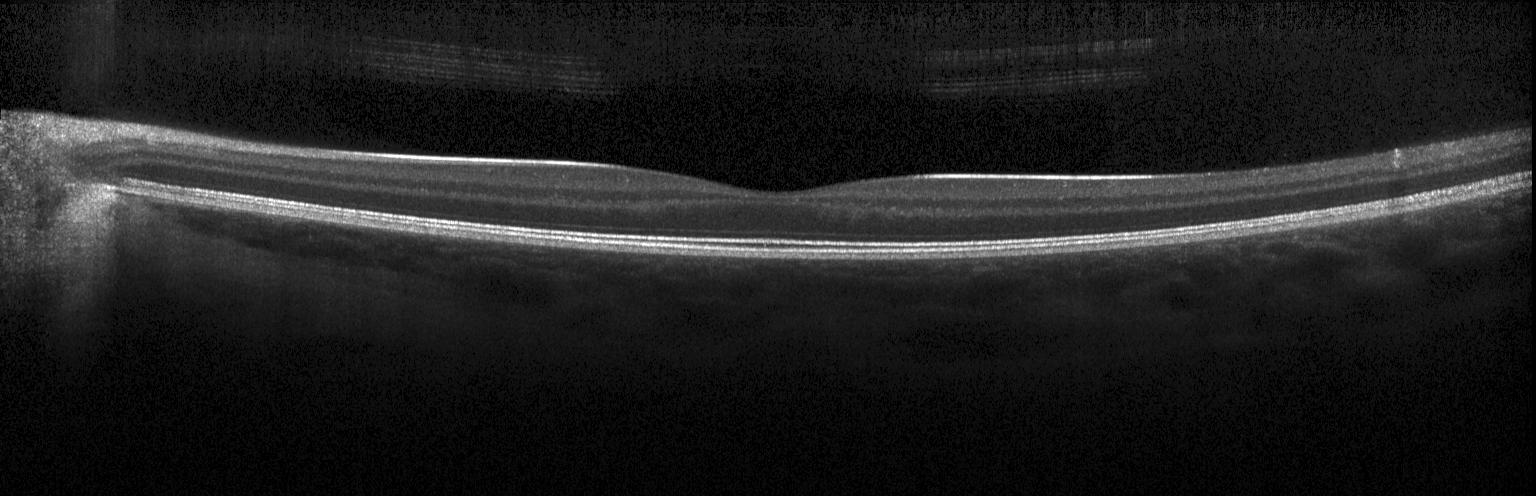
Finding: no choroidal neovascularization, no diabetic macular edema, and no drusen.